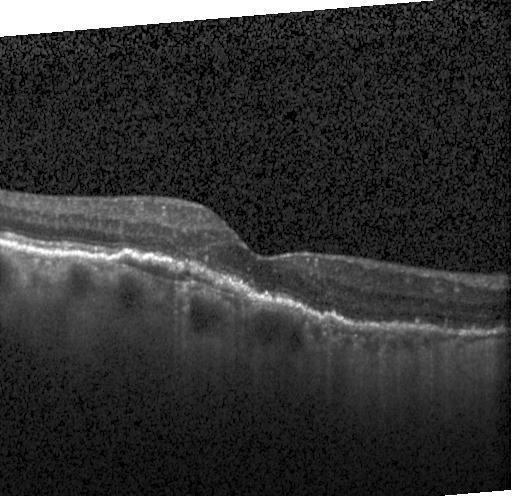
Finding: a choroidal neovascular membrane.